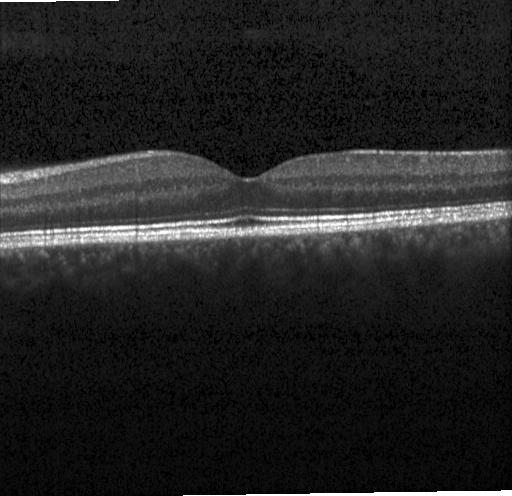
OCT line scan
Assessment: neither CNV, DME, nor drusen.